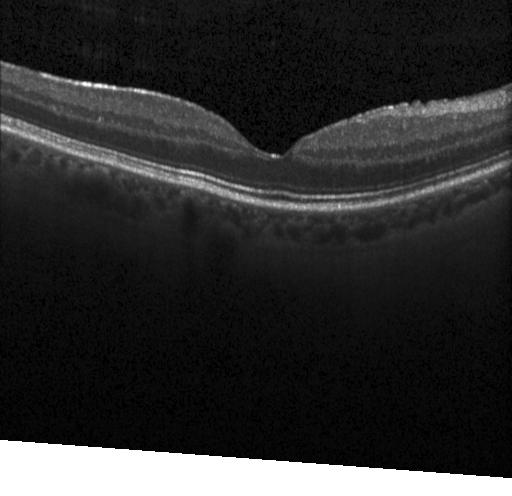 OCT line scan · instrument: Heidelberg Spectralis · spectral-domain optical coherence tomography. Impression: no choroidal neovascularization, diabetic macular edema, or drusen.